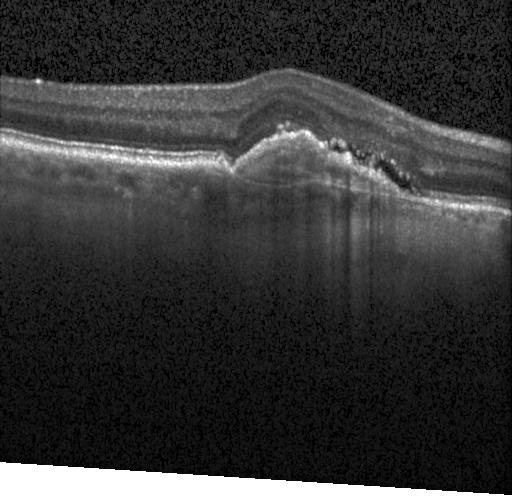
OCT B-scan showing a choroidal neovascular membrane.